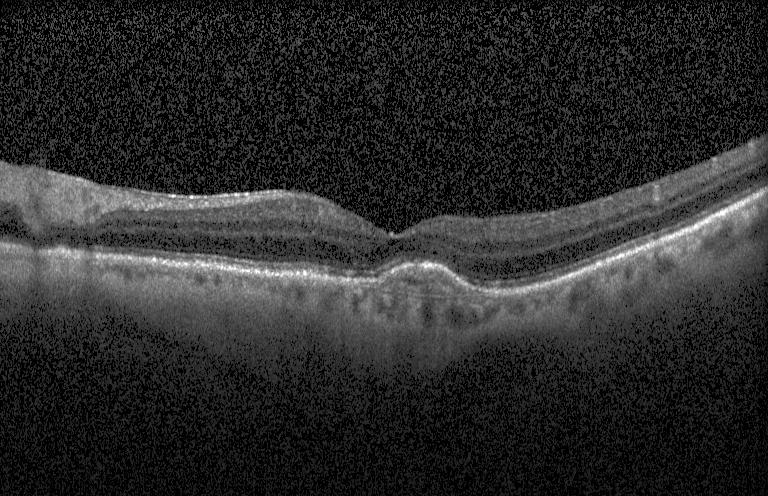

Optical coherence tomography scan, SD-OCT, horizontal scan through the fovea, acquired on a Heidelberg Spectralis
Diagnosis: choroidal neovascularization.